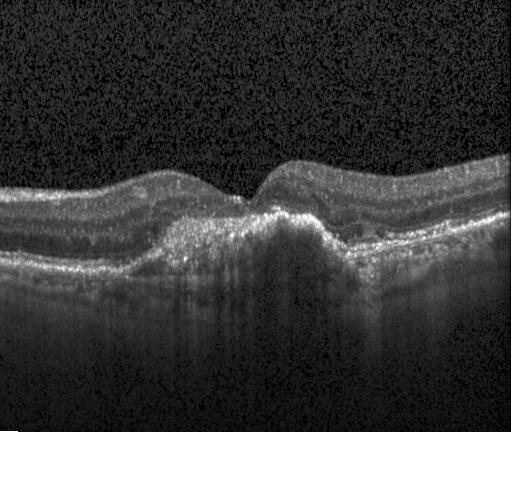
Fovea-centered · retinal OCT cross-section · spectral-domain optical coherence tomography · Heidelberg Spectralis — This B-scan demonstrates choroidal neovascularization.